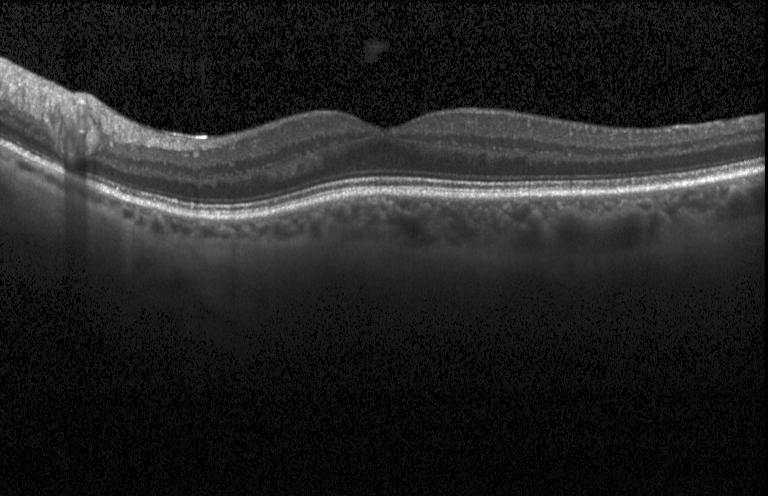 Heidelberg Spectralis, optical coherence tomography B-scan, spectral-domain optical coherence tomography
Assessment: no choroidal neovascularization, no diabetic macular edema, and no drusen.